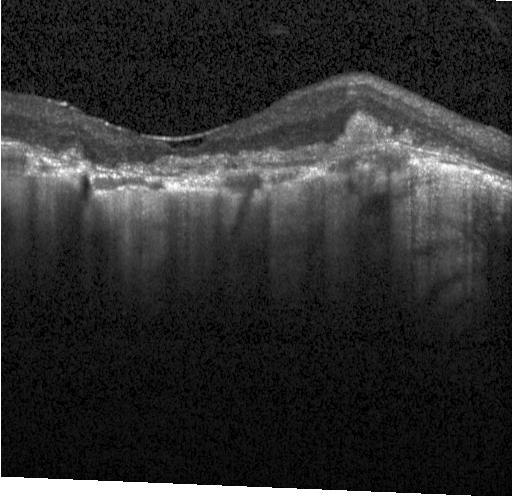 Acquired on a Heidelberg Spectralis · macular scan · spectral-domain OCT · retinal OCT B-scan — Assessment: choroidal neovascularization (CNV).